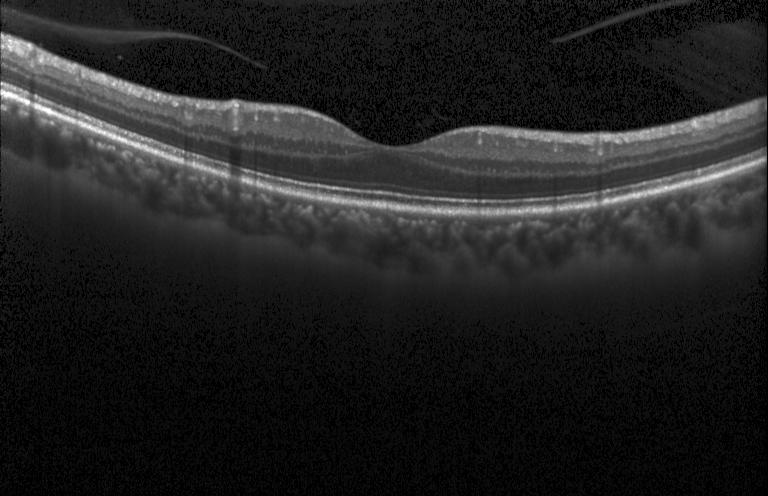
OCT line scan, spectral-domain OCT, instrument: Heidelberg Spectralis, horizontal scan through the fovea.
Macular OCT: no choroidal neovascularization, no diabetic macular edema, and no drusen.